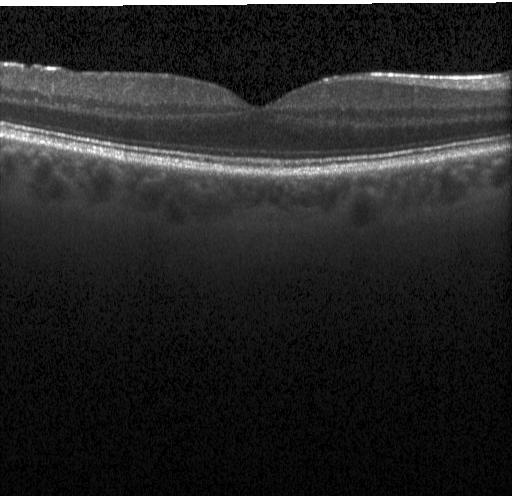
Impression: no choroidal neovascularization, no diabetic macular edema, and no drusen.